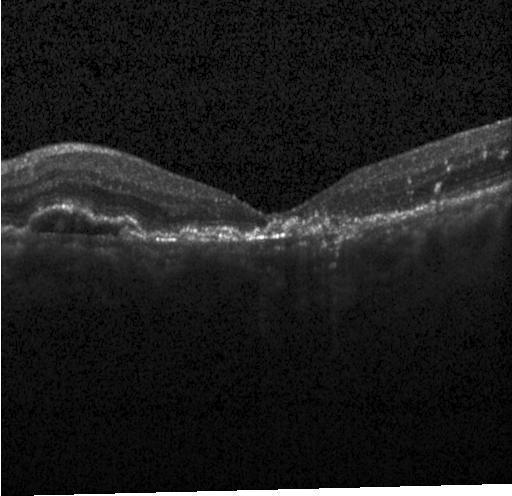 Optical coherence tomography scan
This B-scan demonstrates a choroidal neovascular membrane.